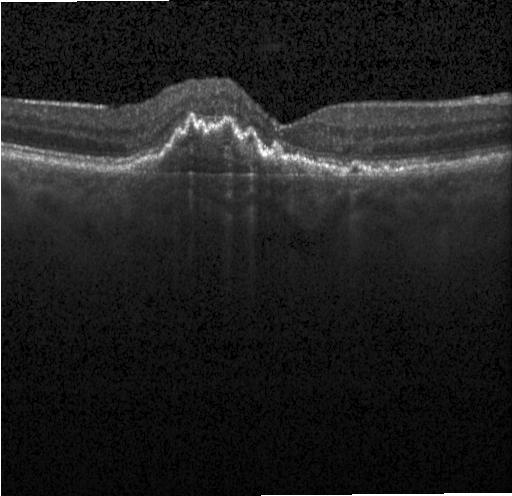 OCT B-scan. The scan shows a choroidal neovascular membrane.